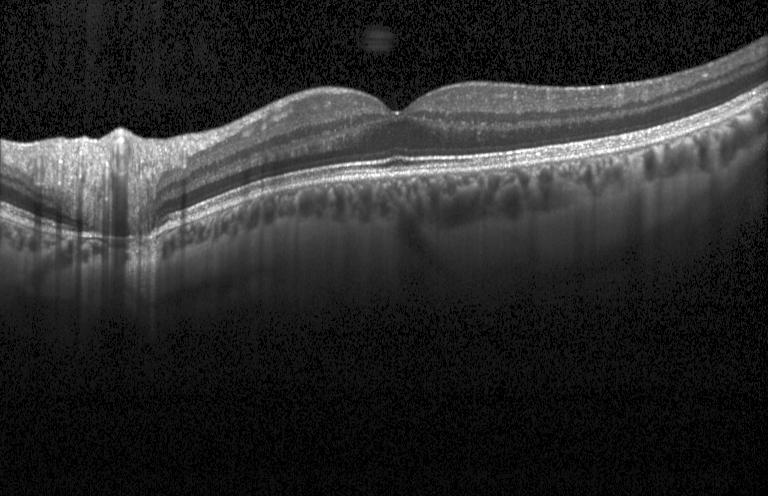
Spectral-domain OCT, optical coherence tomography scan.
Finding: no evidence of choroidal neovascularization, diabetic macular edema, or drusen.